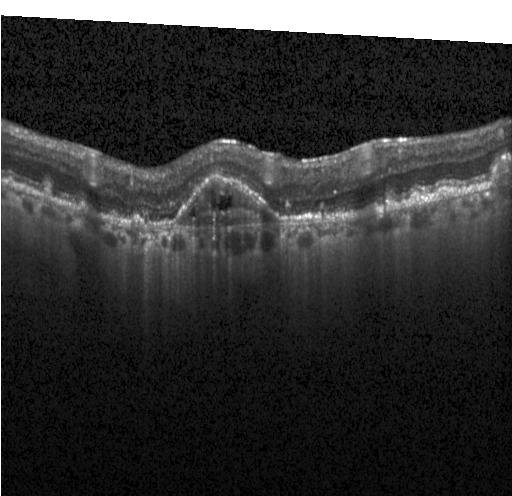
Diagnosis: a choroidal neovascular membrane.